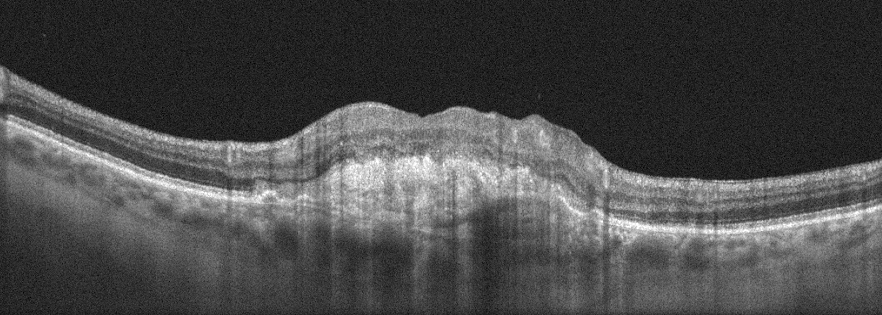
OCT line scan; OS.
Assessment: AMD.